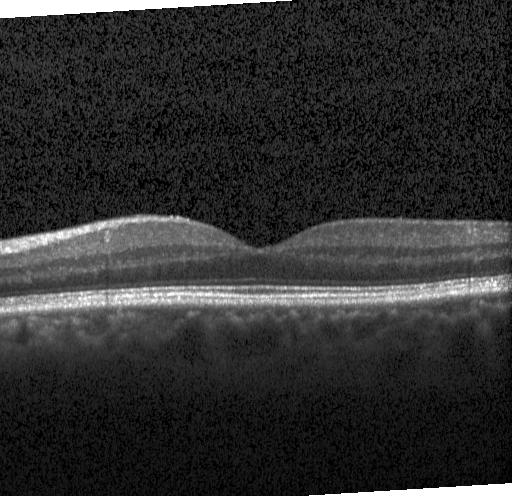 Retinal OCT cross-section showing neither choroidal neovascularization, diabetic macular edema, nor drusen.